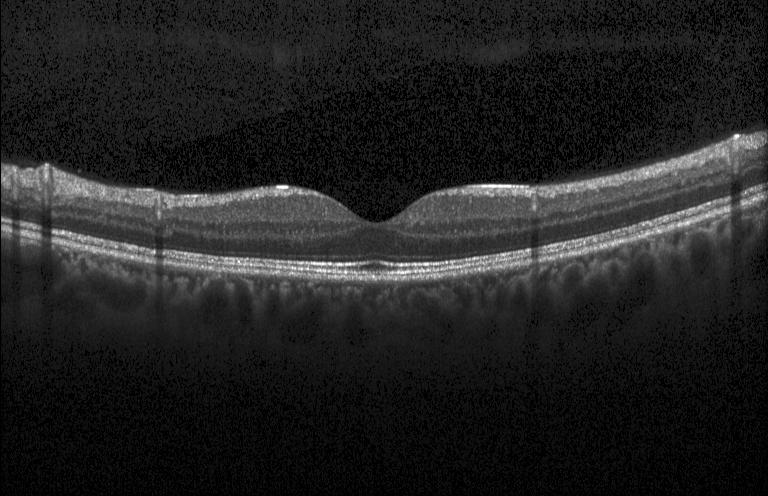
The scan shows no choroidal neovascularization, diabetic macular edema, or drusen.